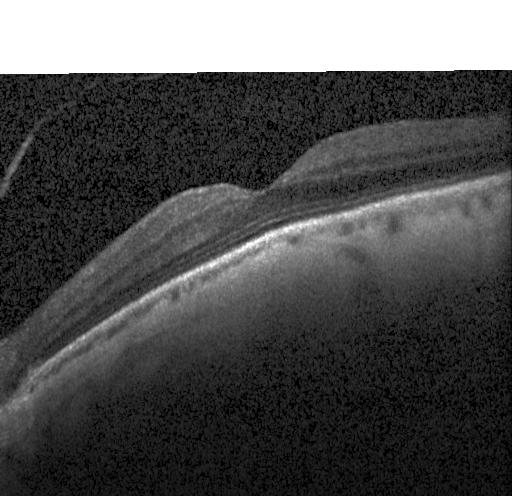

Impression: no choroidal neovascularization, diabetic macular edema, or drusen.